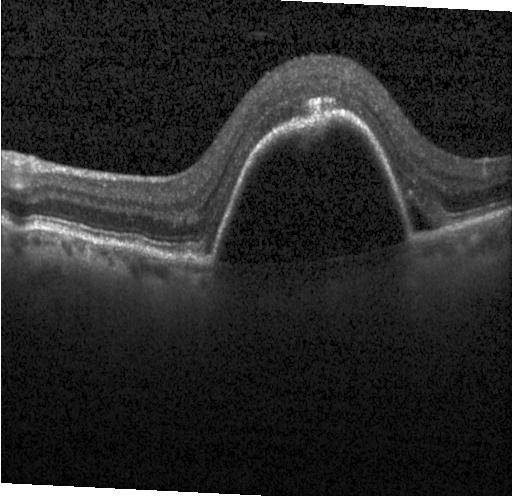
Optical coherence tomography scan.
Impression: CNV.